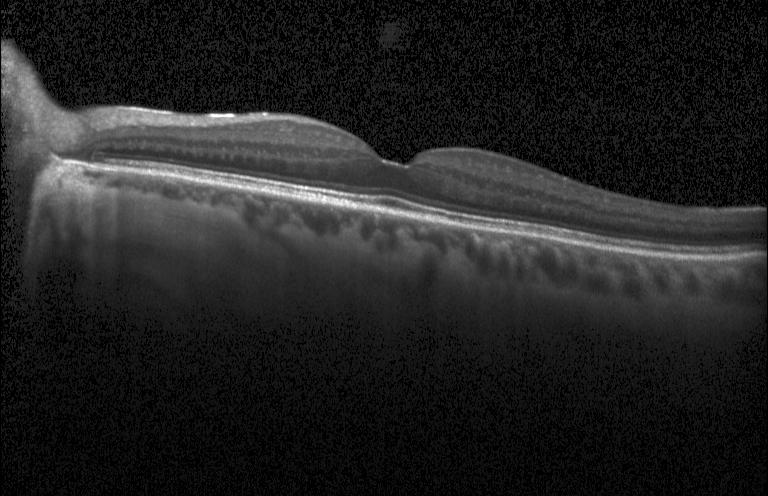 OCT finding: neither choroidal neovascularization, diabetic macular edema, nor drusen.